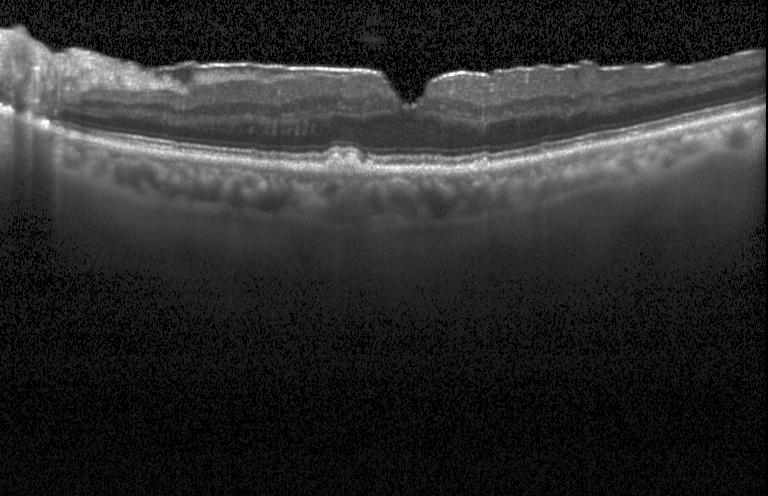

Assessment: multiple drusen.